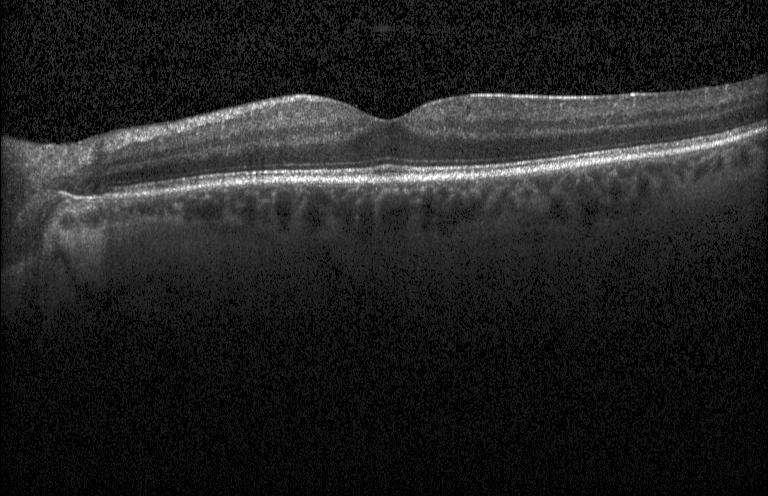
No choroidal neovascularization, diabetic macular edema, or drusen.